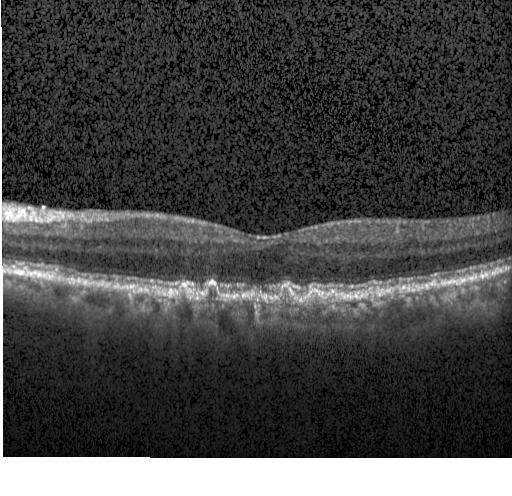 Fovea-centered · optical coherence tomography scan — Impression: drusen.